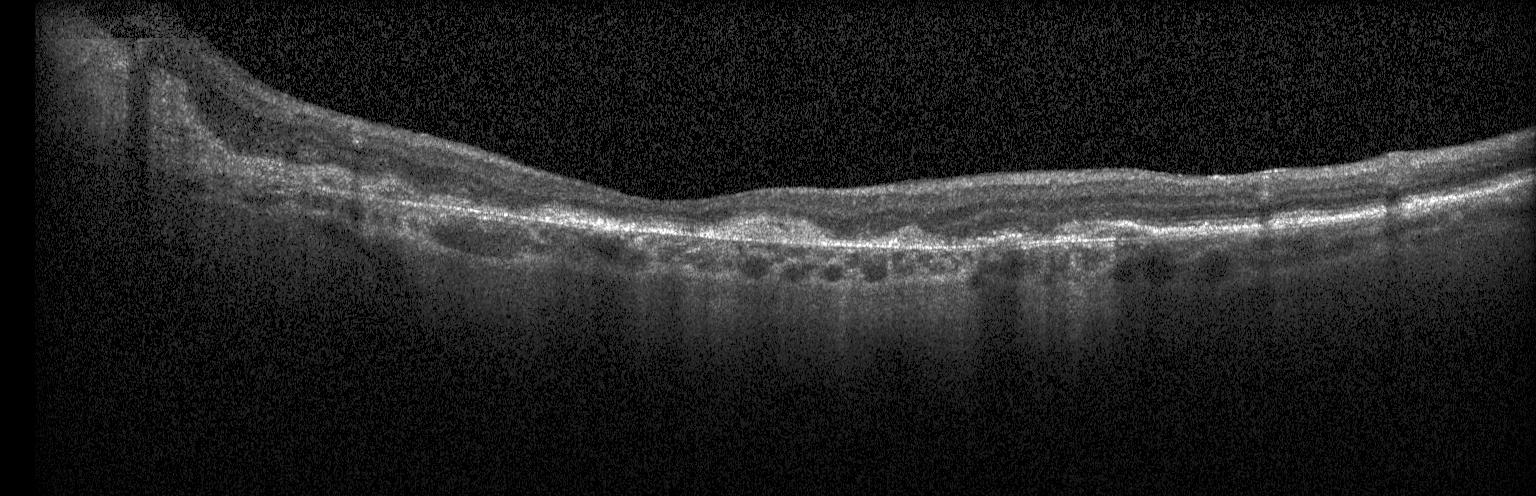
Assessment: choroidal neovascularization.